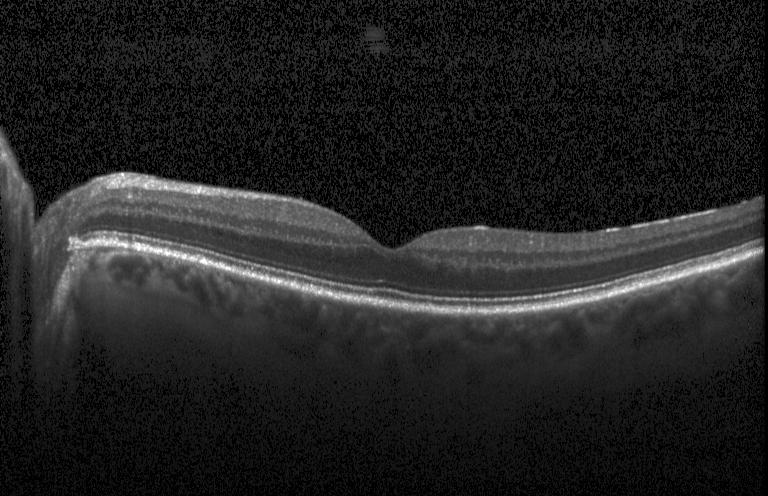 Optical coherence tomography B-scan
This B-scan demonstrates no choroidal neovascularization, no diabetic macular edema, and no drusen.